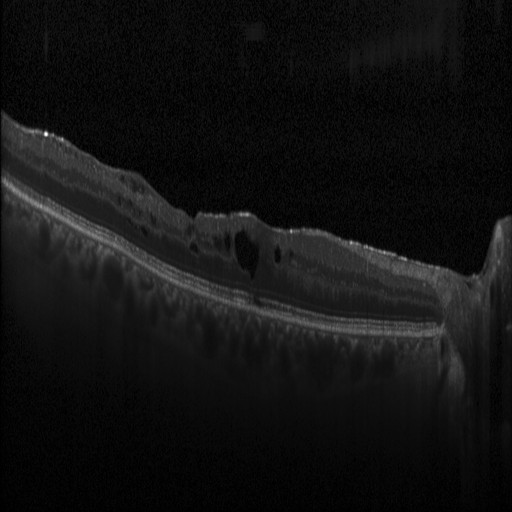 Instrument: Heidelberg Spectralis; macular scan; OCT B-scan; spectral-domain OCT — Diagnosis: DME.